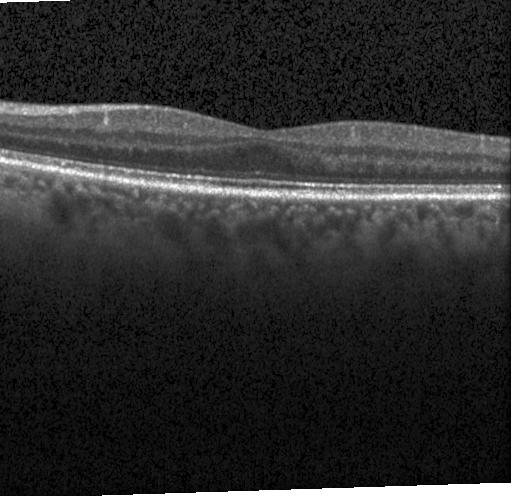 Retinal OCT cross-section; macular scan; Heidelberg Spectralis; spectral-domain optical coherence tomography.
Impression: no evidence of CNV, DME, or drusen.